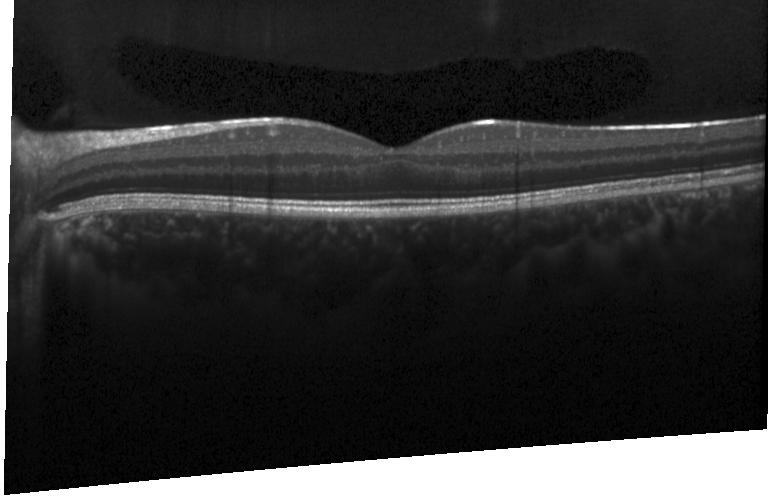 Fovea-centered; optical coherence tomography scan — Finding: neither choroidal neovascularization, diabetic macular edema, nor drusen.